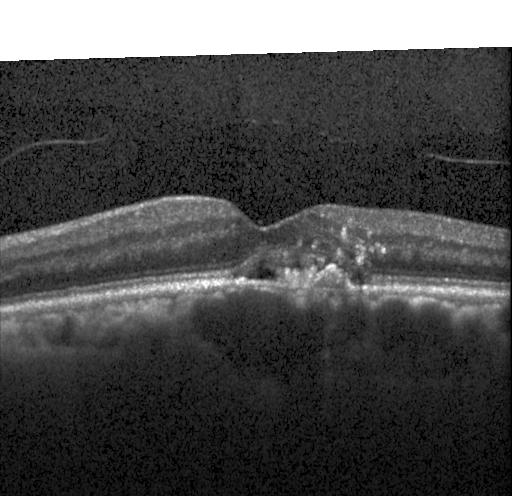

Finding: a choroidal neovascular membrane.